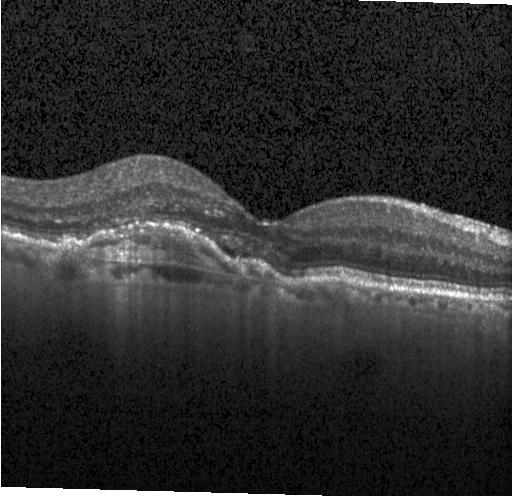
A choroidal neovascular membrane.